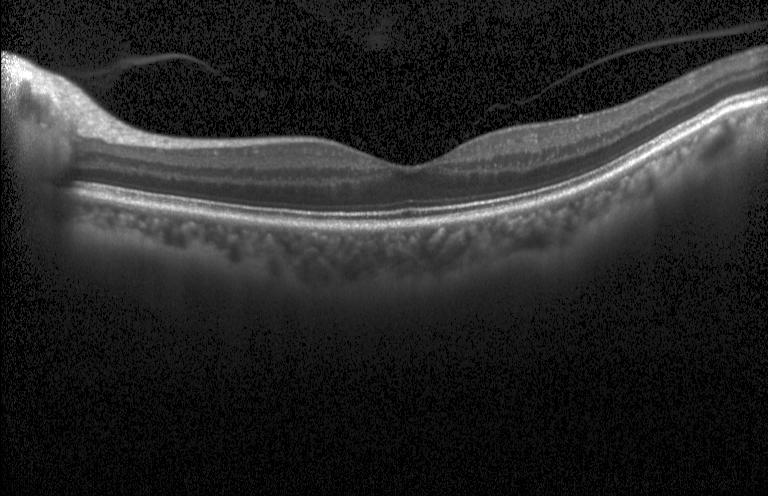

OCT B-scan
Finding: no CNV, no DME, and no drusen.